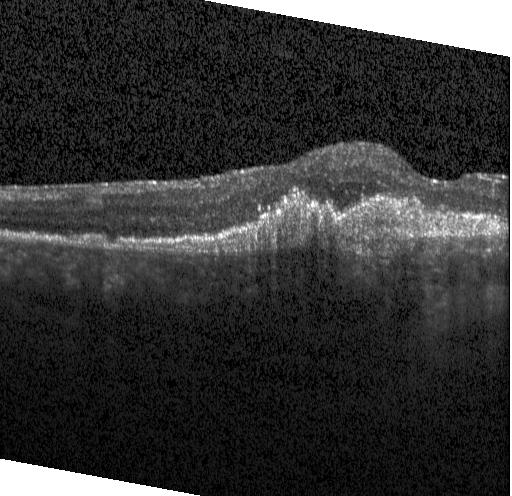 OCT line scan.
Choroidal neovascularization (CNV).